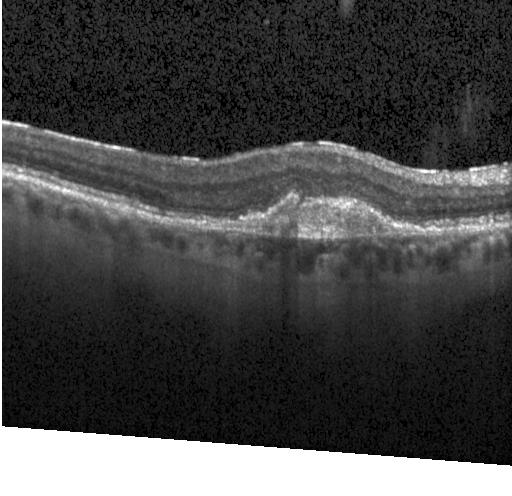

Through the macula; acquired on a Heidelberg Spectralis; optical coherence tomography scan; spectral-domain optical coherence tomography.
Diagnosis: choroidal neovascularization.